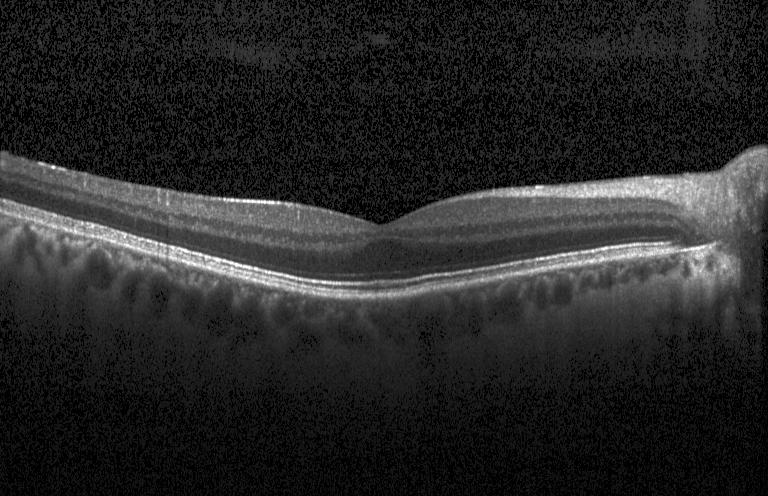
Fovea-centered, Heidelberg Spectralis OCT system, OCT line scan
The scan shows no choroidal neovascularization, no diabetic macular edema, and no drusen.